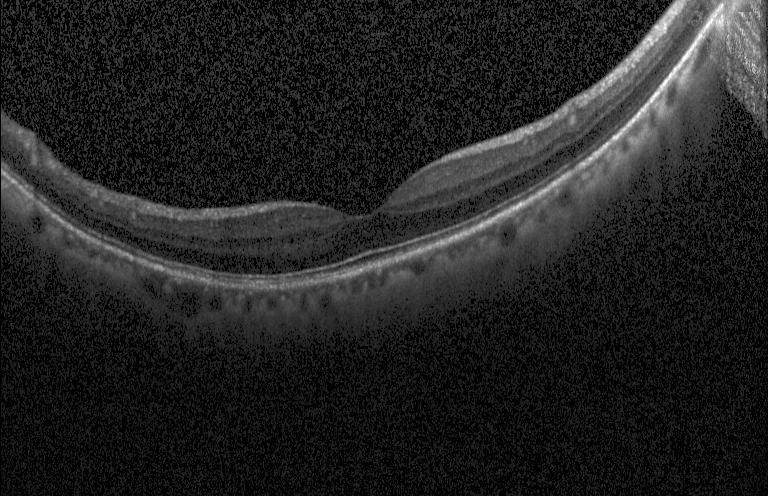 Finding: no choroidal neovascularization, no diabetic macular edema, and no drusen.